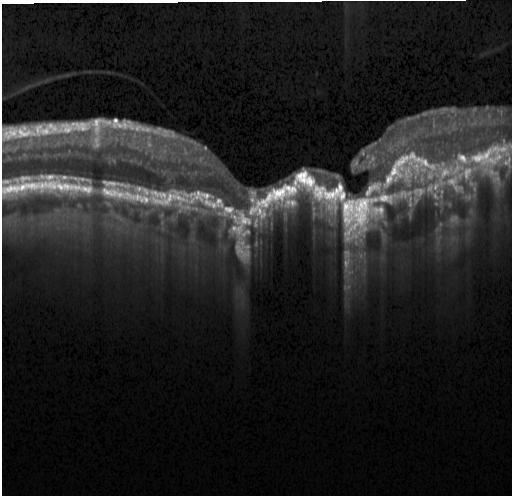
Retinal OCT B-scan.
Diagnosis: a choroidal neovascular membrane.